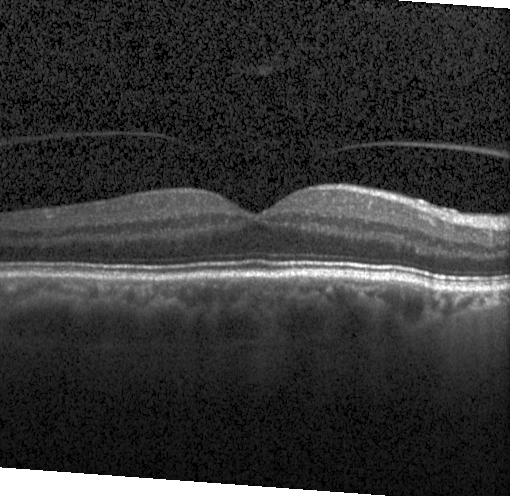 Spectral-domain optical coherence tomography. Heidelberg Spectralis. OCT line scan
Neither choroidal neovascularization, diabetic macular edema, nor drusen.